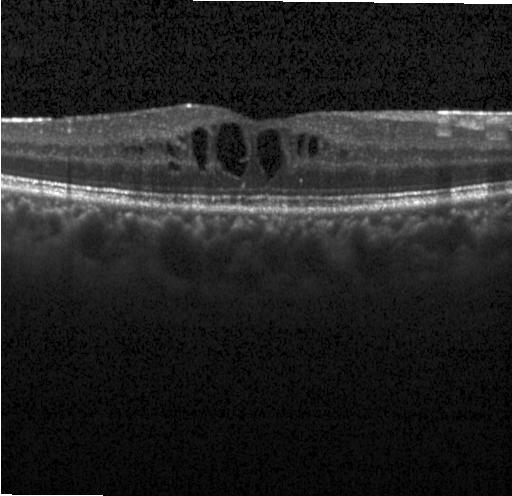
Dx: DME.